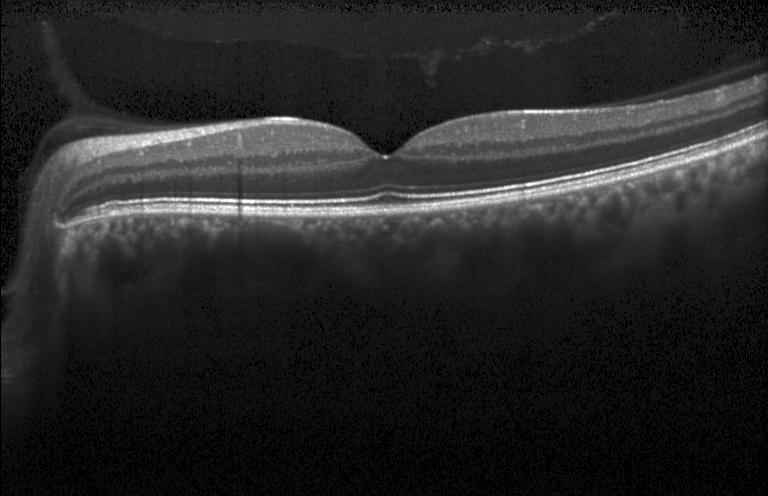

Heidelberg Spectralis · retinal OCT cross-section · through the macula · spectral-domain optical coherence tomography
This B-scan demonstrates no choroidal neovascularization, no diabetic macular edema, and no drusen.